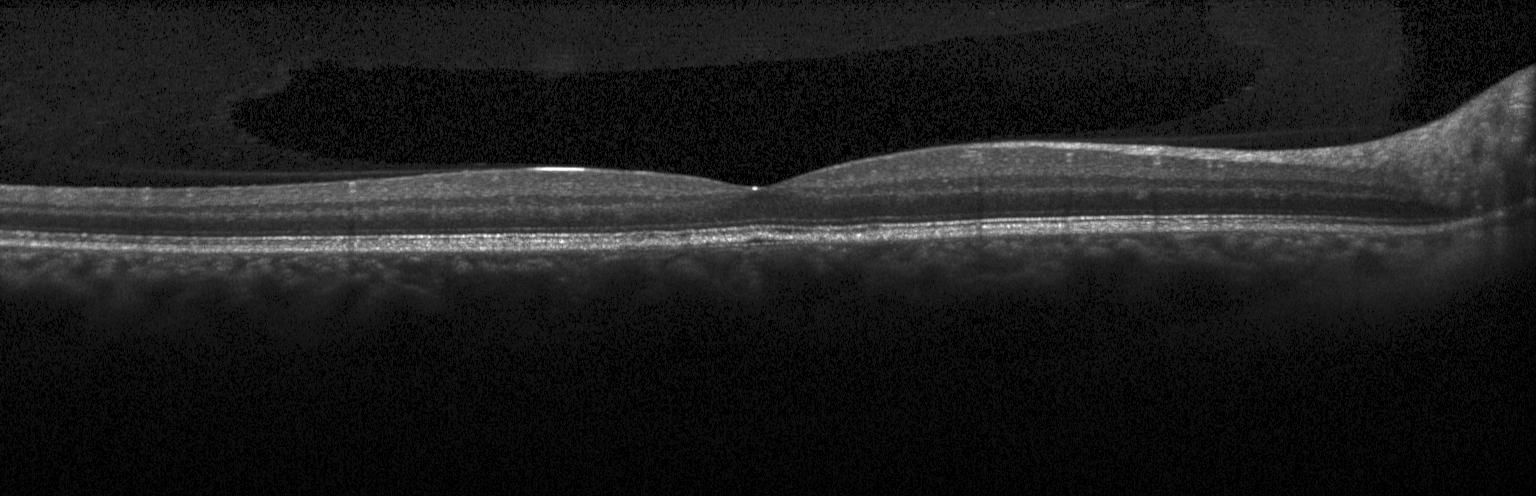 Impression: no evidence of CNV, DME, or drusen.